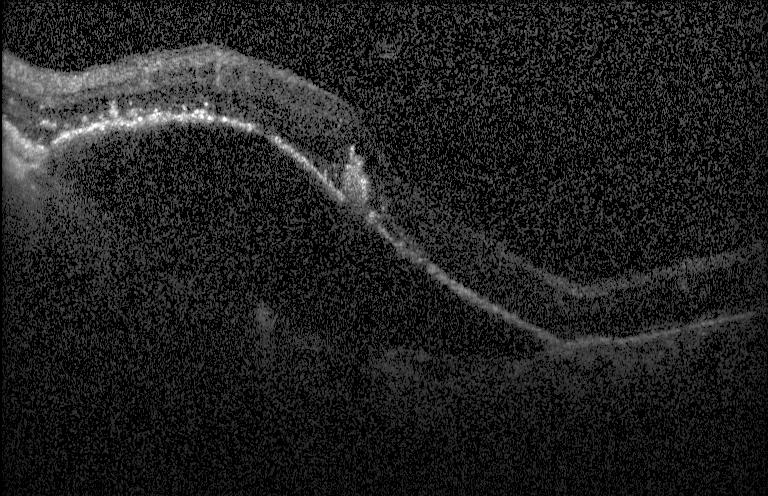 Retinal OCT cross-section. Spectral-domain optical coherence tomography. Heidelberg Spectralis OCT system
This B-scan demonstrates CNV.